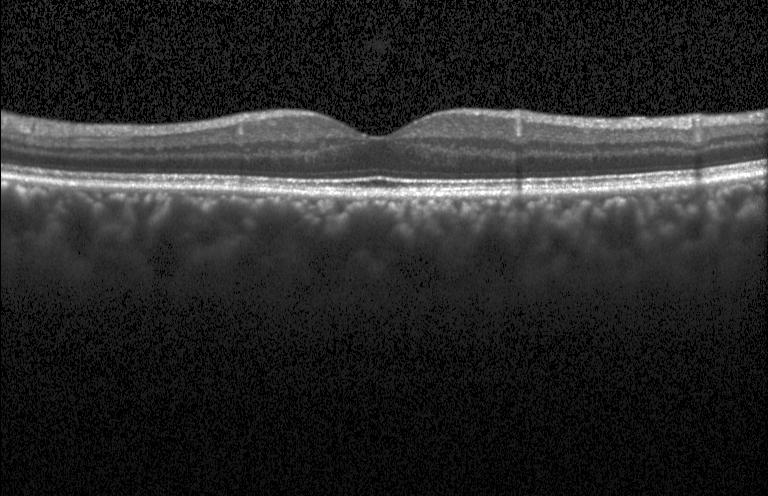 This B-scan demonstrates neither choroidal neovascularization, diabetic macular edema, nor drusen.